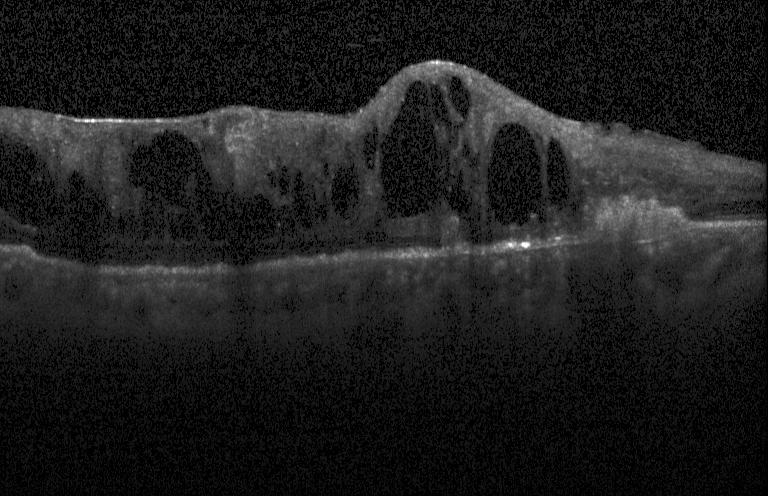 Macular scan, SD-OCT, OCT line scan, acquired on a Heidelberg Spectralis. Finding: choroidal neovascularization.